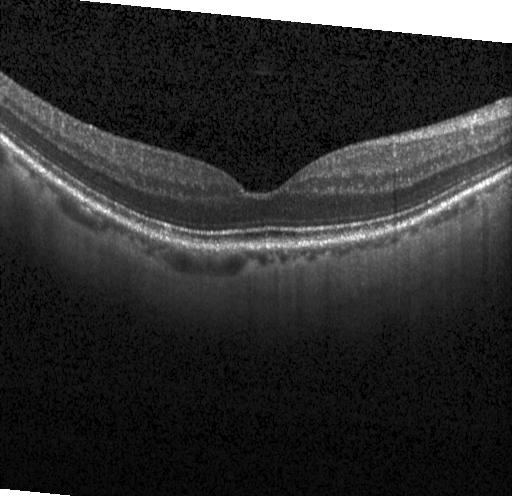
Optical coherence tomography B-scan · instrument: Heidelberg Spectralis.
OCT finding: no evidence of choroidal neovascularization, diabetic macular edema, or drusen.